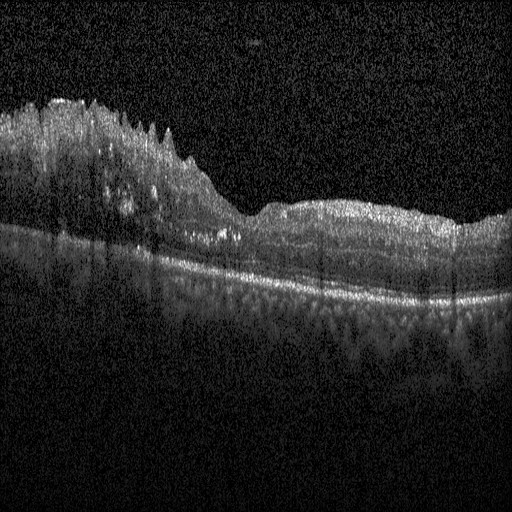 Instrument: Heidelberg Spectralis; optical coherence tomography B-scan; spectral-domain OCT; through the macula.
Assessment: diabetic macular edema.